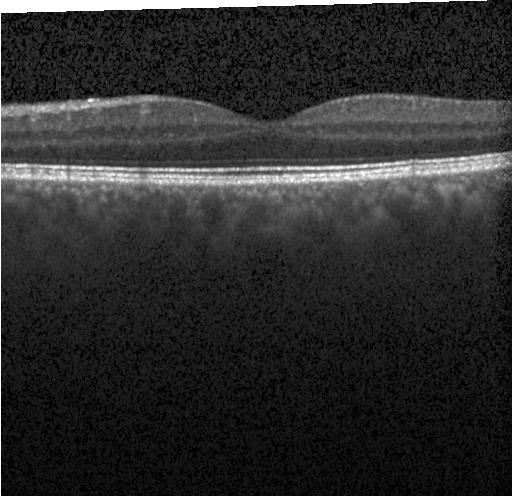 Spectral-domain OCT, optical coherence tomography scan, acquired on a Heidelberg Spectralis, horizontal scan through the fovea — No choroidal neovascularization, no diabetic macular edema, and no drusen.